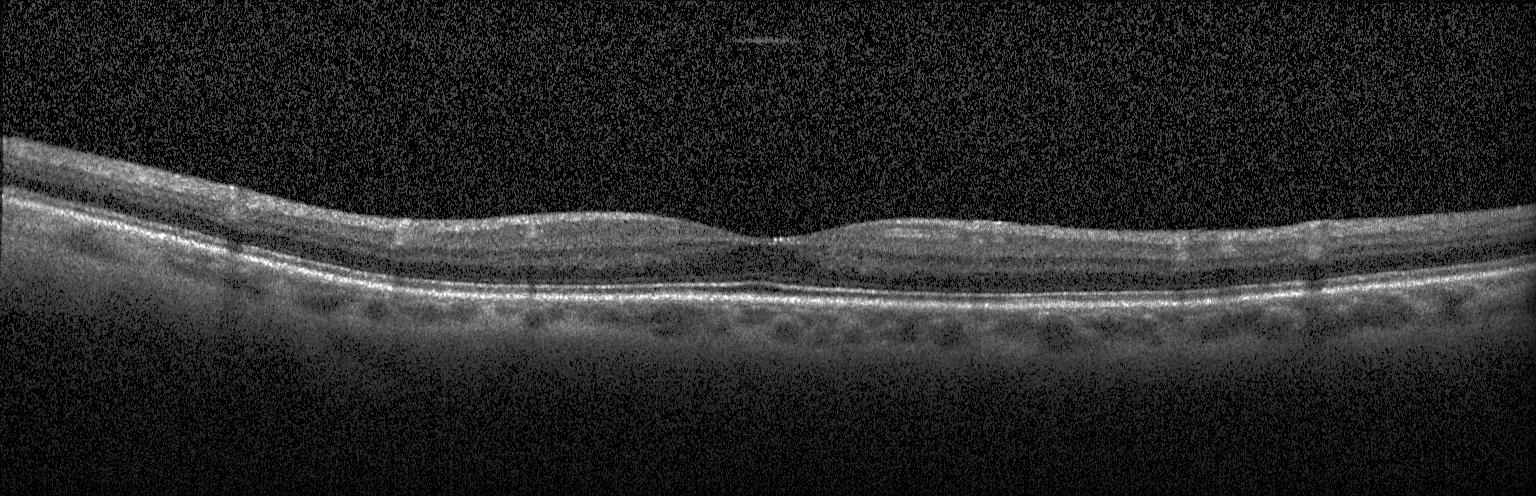 Spectral-domain optical coherence tomography. Through the macula. Instrument: Heidelberg Spectralis. Retinal OCT B-scan. Dx: no choroidal neovascularization, diabetic macular edema, or drusen.